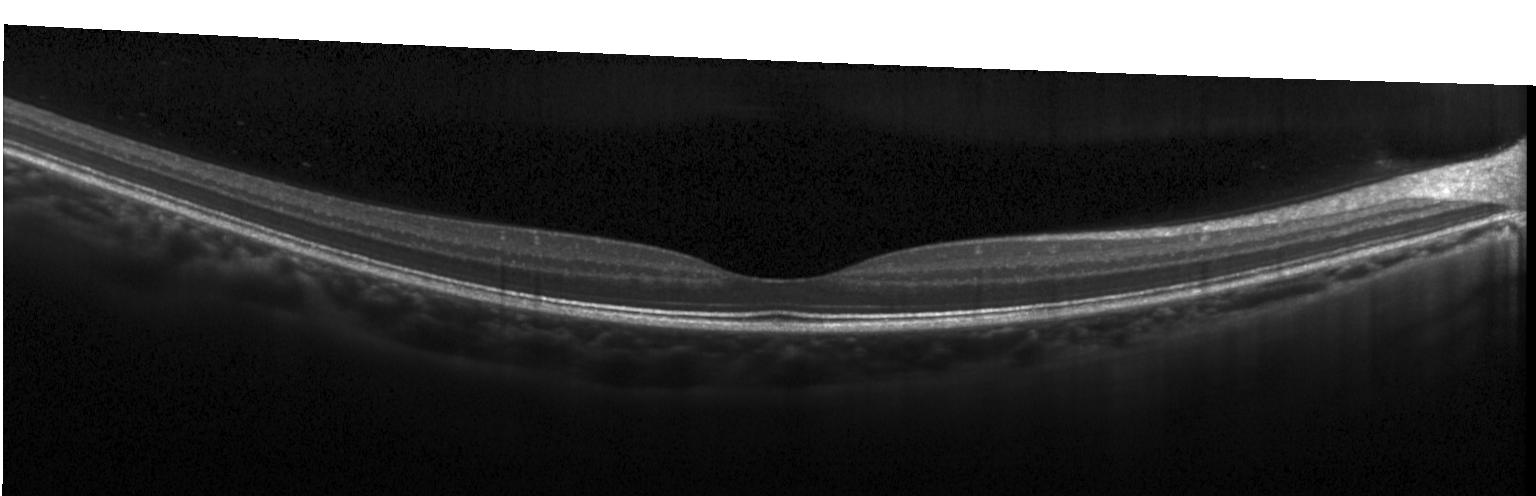

The scan shows no choroidal neovascularization, diabetic macular edema, or drusen.